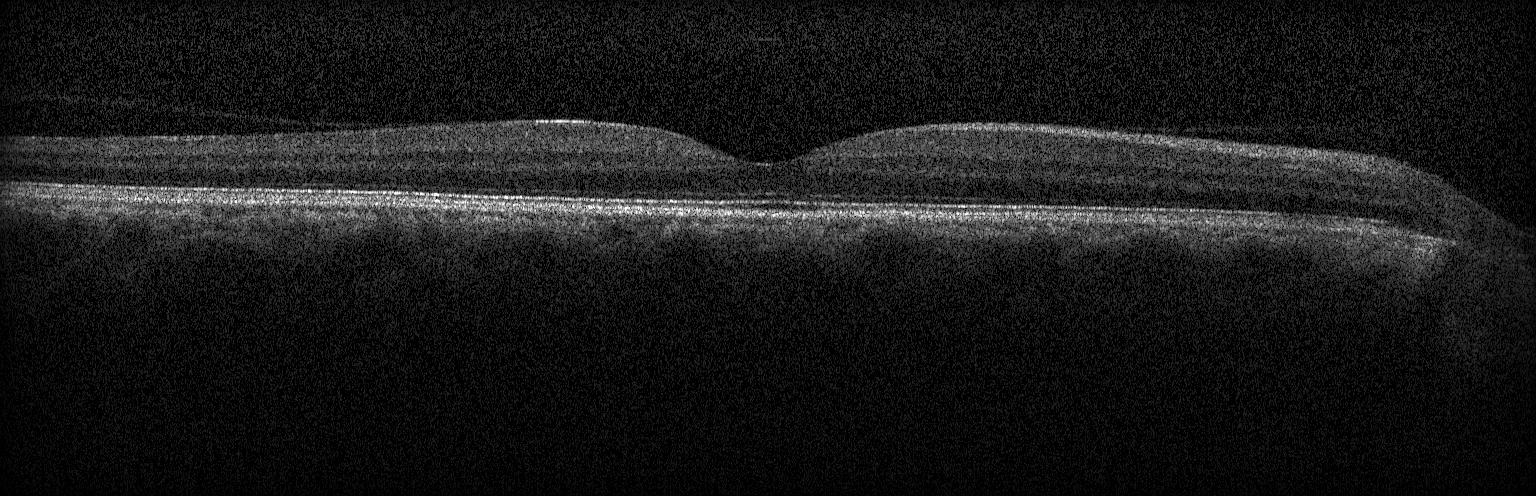 Retinal OCT cross-section · spectral-domain OCT · Heidelberg Spectralis · macular scan
OCT finding: no CNV, no DME, and no drusen.